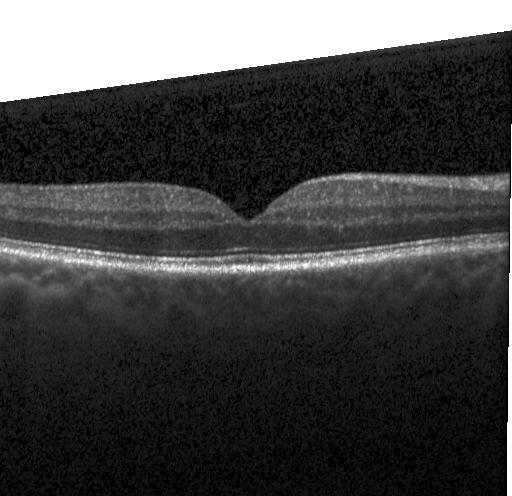

Retinal OCT cross-section, instrument: Heidelberg Spectralis. Assessment: neither CNV, DME, nor drusen.